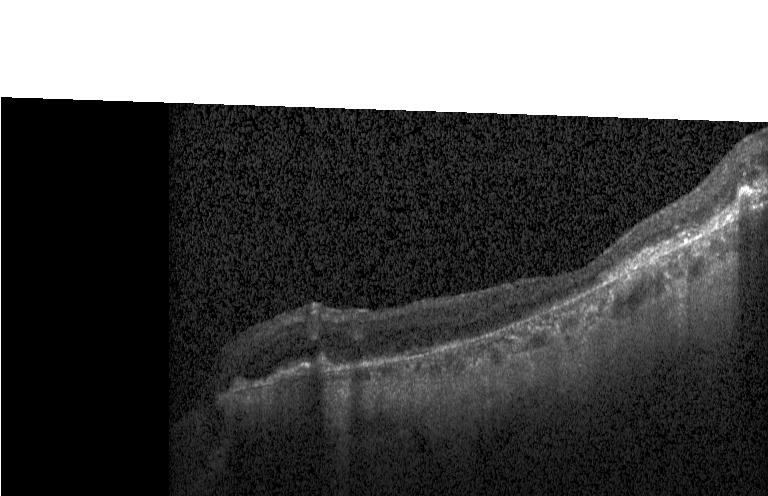

OCT B-scan; Heidelberg Spectralis OCT system; fovea-centered; spectral-domain OCT.
Impression: choroidal neovascularization (CNV).